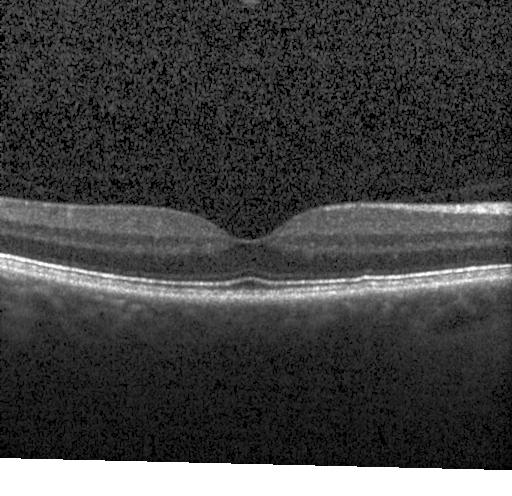
Diagnosis: no evidence of choroidal neovascularization, diabetic macular edema, or drusen.